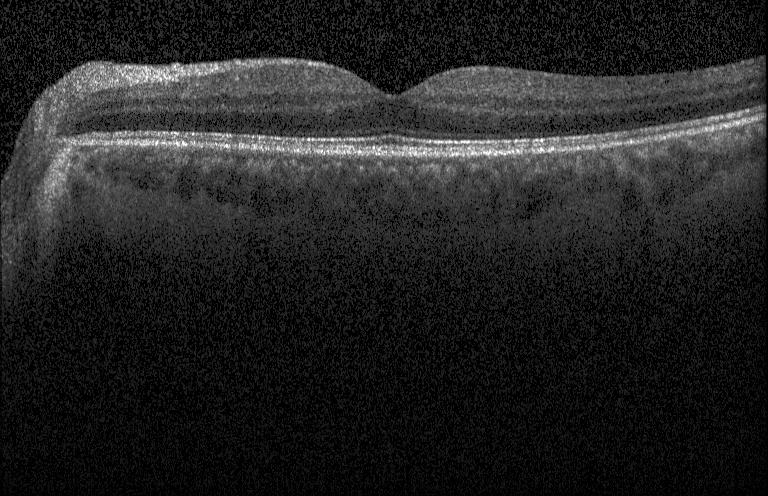 OCT B-scan
Finding: no choroidal neovascularization, no diabetic macular edema, and no drusen.